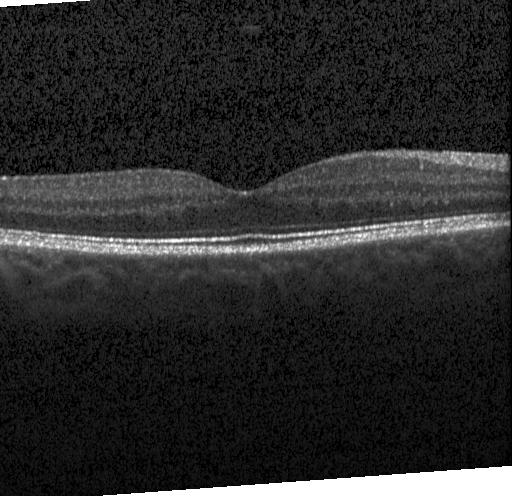 OCT line scan. Finding: no choroidal neovascularization, diabetic macular edema, or drusen.